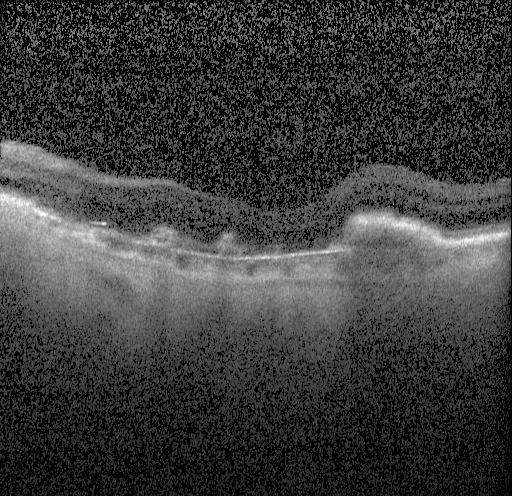

Macular OCT: choroidal neovascularization.